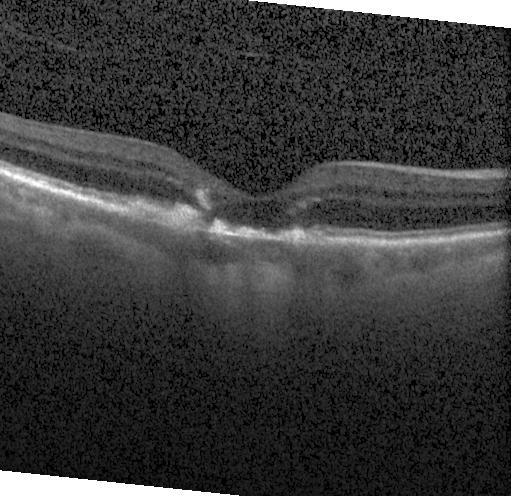

Optical coherence tomography scan.
A choroidal neovascular membrane.